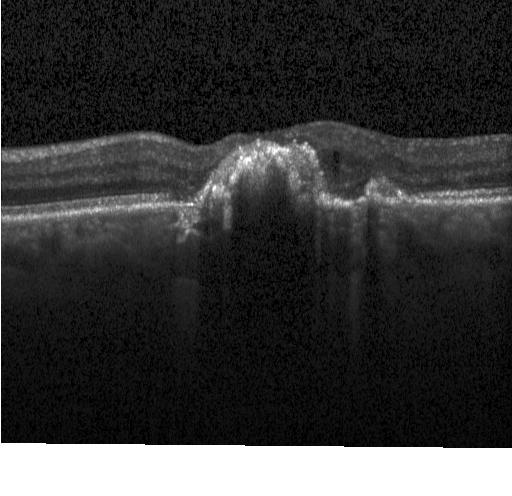

Dx: a choroidal neovascular membrane.